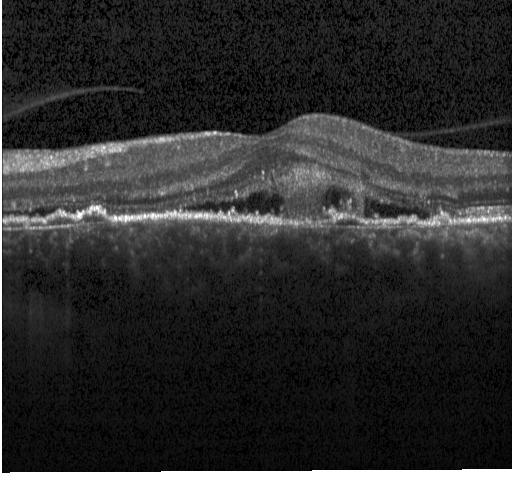 OCT B-scan showing choroidal neovascularization (CNV).